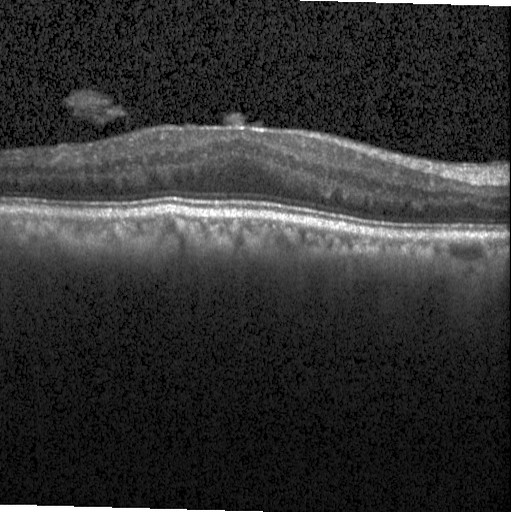 Spectral-domain OCT B-scan: diabetic macular edema (DME).